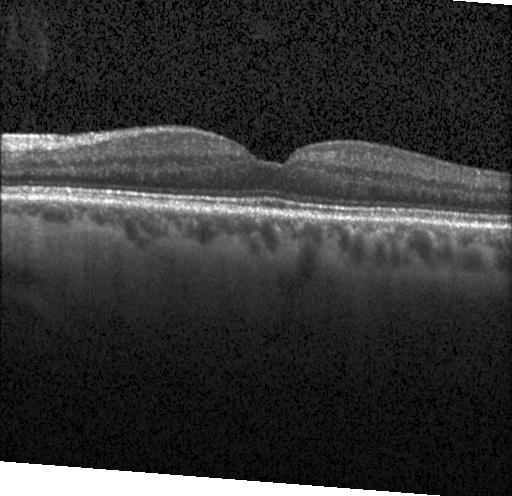
Horizontal scan through the fovea, retinal OCT cross-section. Finding: no choroidal neovascularization, diabetic macular edema, or drusen.